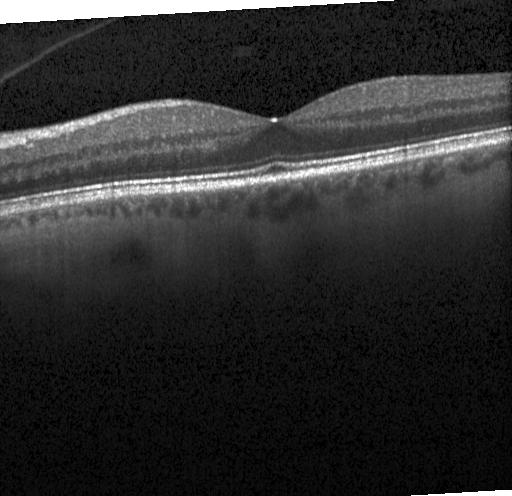
Optical coherence tomography B-scan, SD-OCT, fovea-centered. The scan shows no choroidal neovascularization, no diabetic macular edema, and no drusen.